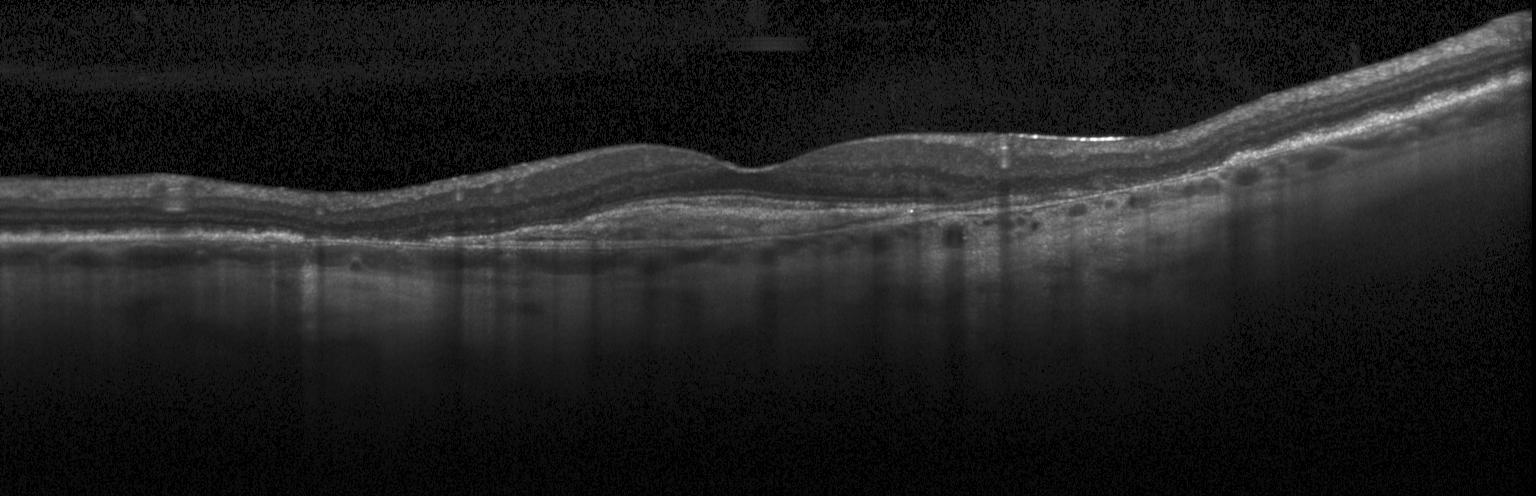 Diagnosis: a choroidal neovascular membrane.